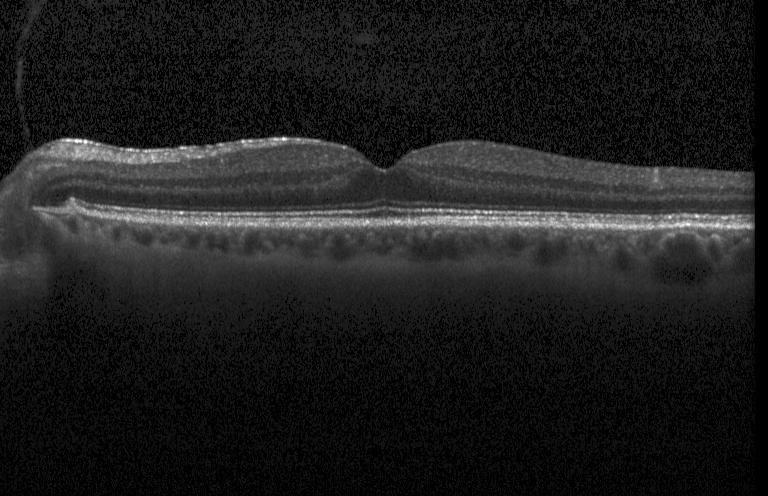
Horizontal scan through the fovea, retinal OCT cross-section, acquired on a Heidelberg Spectralis — Impression: no CNV, no DME, and no drusen.